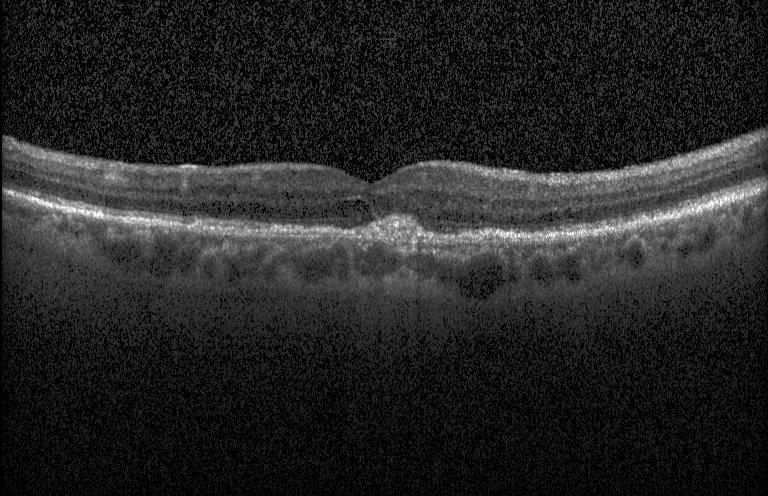 Macular OCT: choroidal neovascularization (CNV).